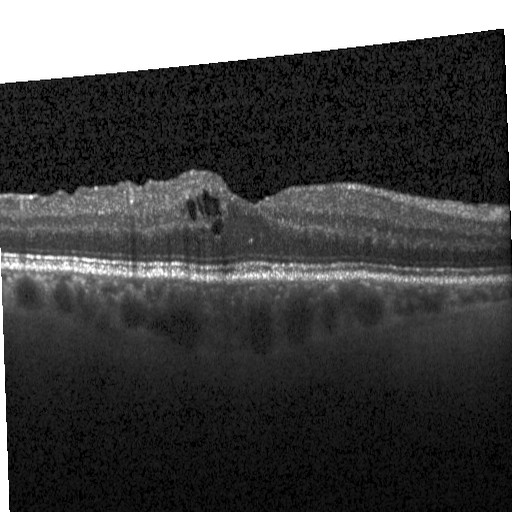
Retinal OCT cross-section; instrument: Heidelberg Spectralis — OCT finding: DME.